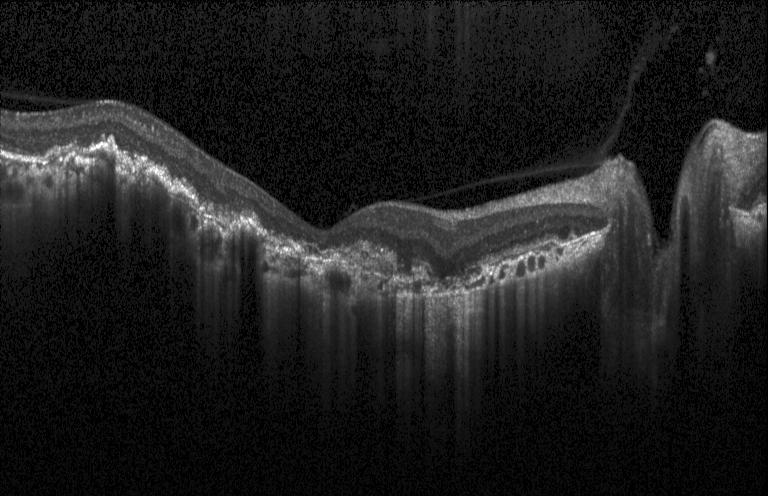 Optical coherence tomography B-scan — Impression: CNV.